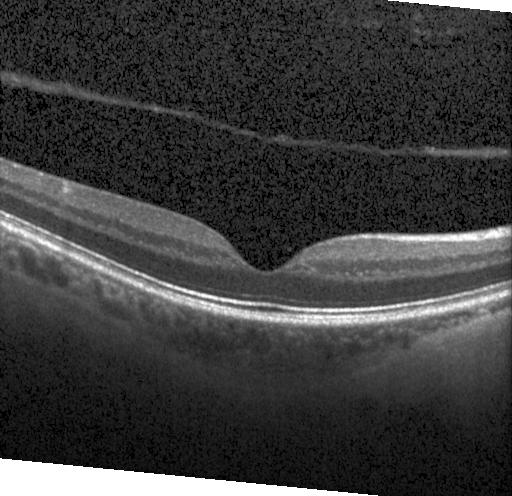

The scan shows neither CNV, DME, nor drusen.